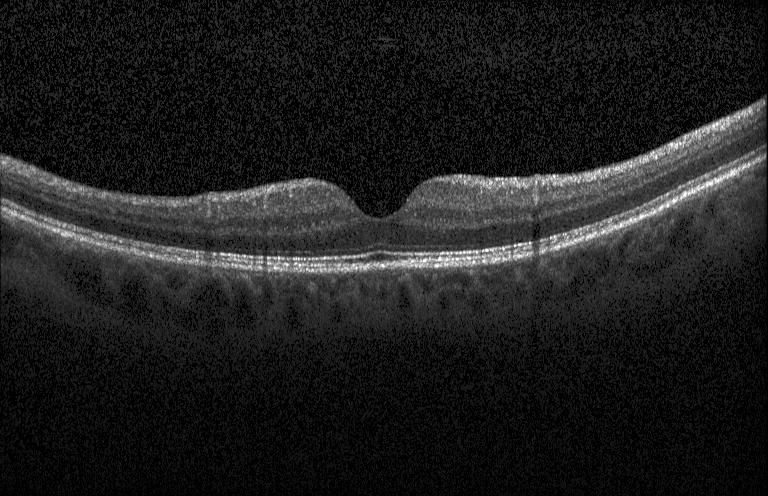 Horizontal scan through the fovea. Spectral-domain OCT. Retinal OCT B-scan. Heidelberg Spectralis
Finding: no choroidal neovascularization, no diabetic macular edema, and no drusen.